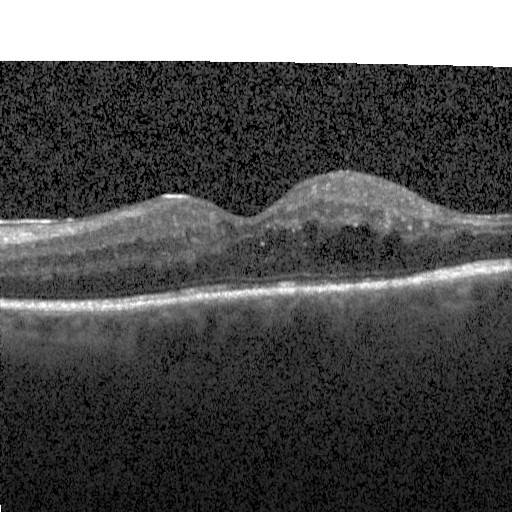 Retinal OCT cross-section showing diabetic macular edema (DME).